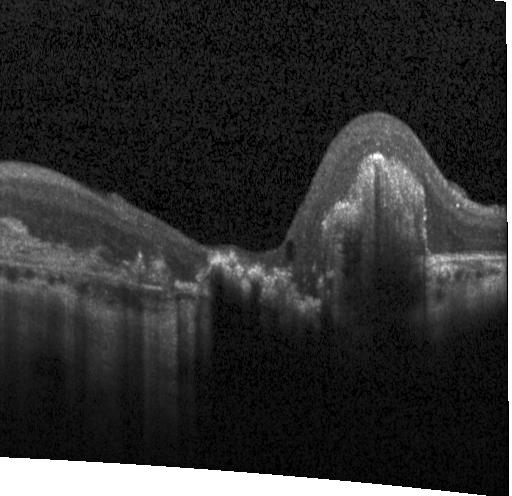
Macular OCT: CNV.